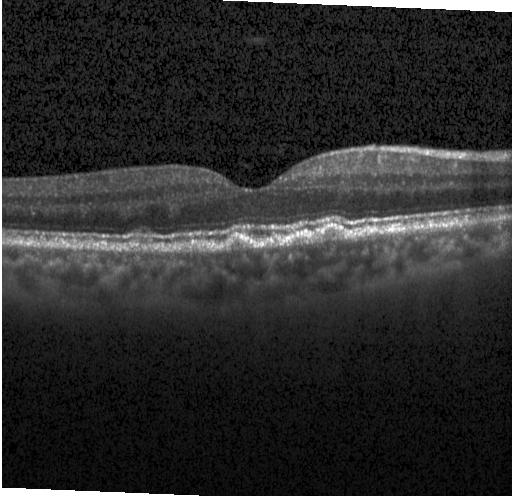 Optical coherence tomography B-scan
This B-scan demonstrates drusen.